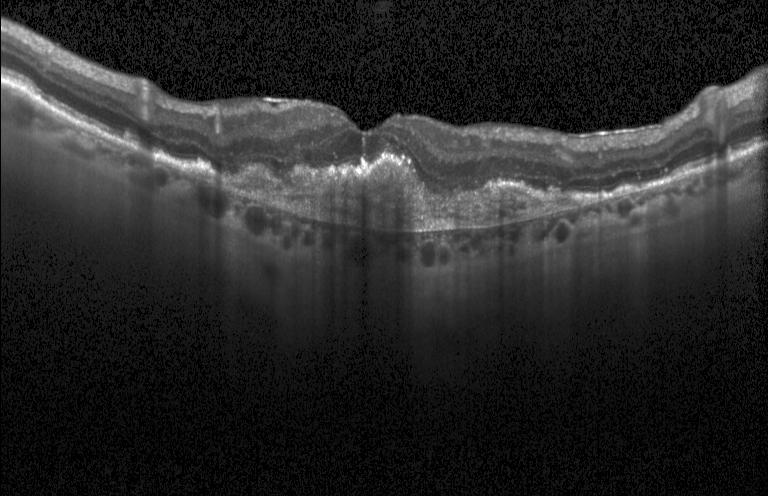

OCT B-scan, spectral-domain optical coherence tomography
Macular OCT: a choroidal neovascular membrane.